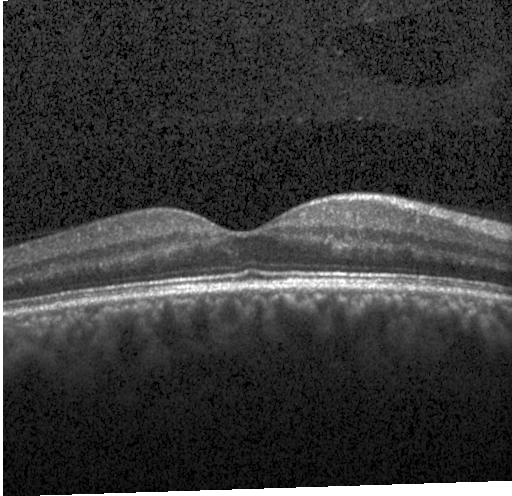

Horizontal scan through the fovea, OCT line scan
Finding: no choroidal neovascularization, no diabetic macular edema, and no drusen.